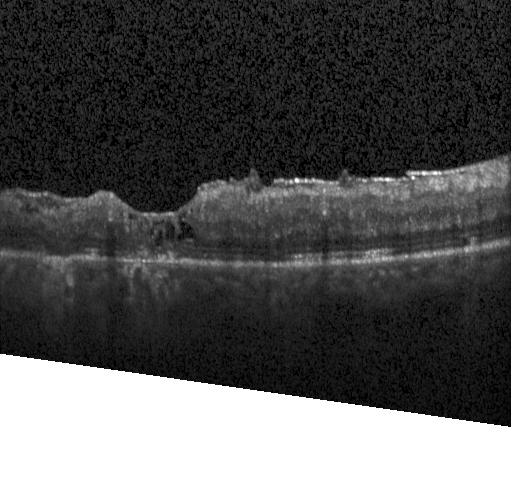

OCT finding: diabetic macular edema.